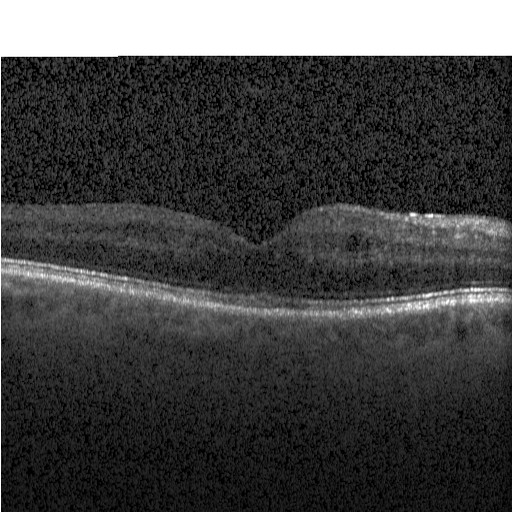

Optical coherence tomography scan
Assessment: DME.